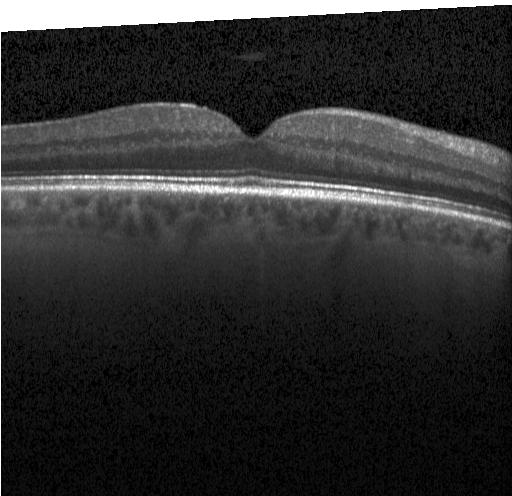

Through the macula, retinal OCT B-scan, Heidelberg Spectralis — Finding: no choroidal neovascularization, diabetic macular edema, or drusen.